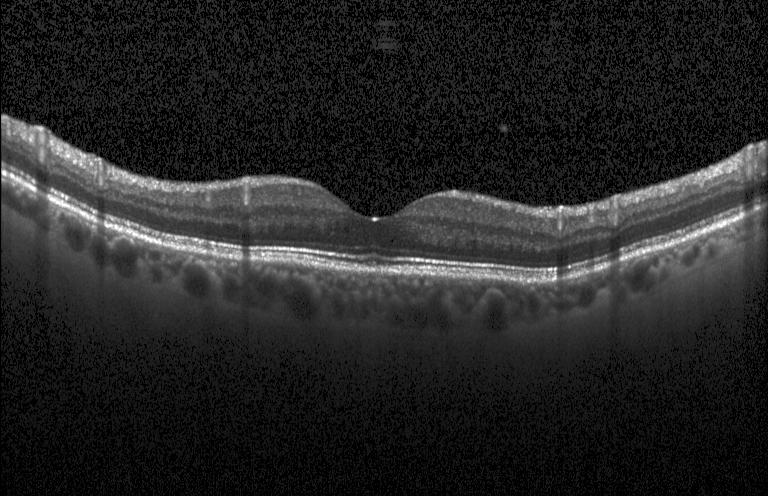
Optical coherence tomography scan; spectral-domain OCT — The scan shows no CNV, DME, or drusen.